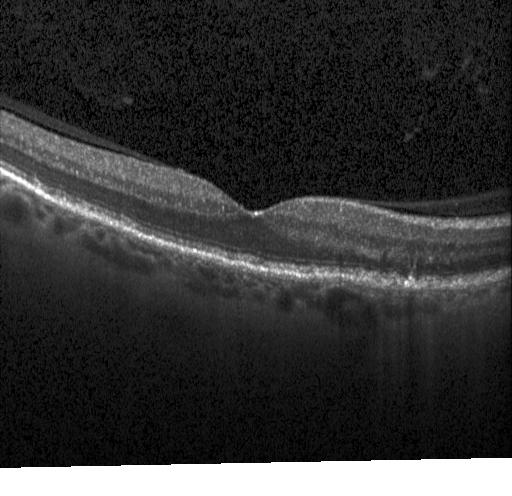
Macular OCT demonstrating no CNV, no DME, and no drusen.